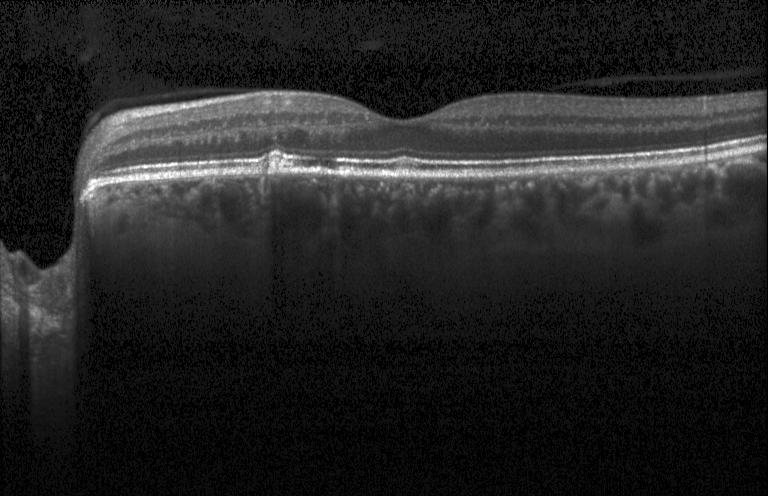

Retinal OCT B-scan · spectral-domain OCT
Finding: drusen.